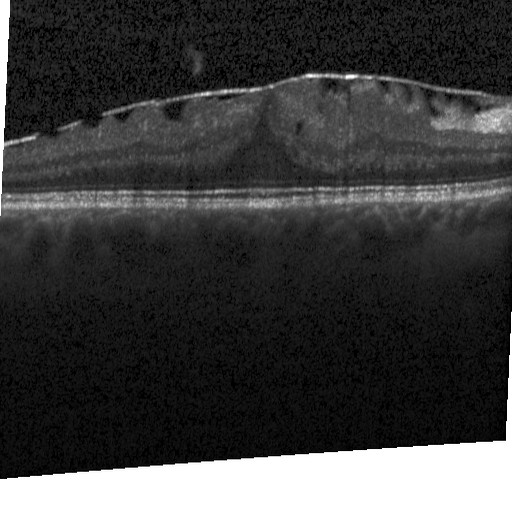 Finding: DME.